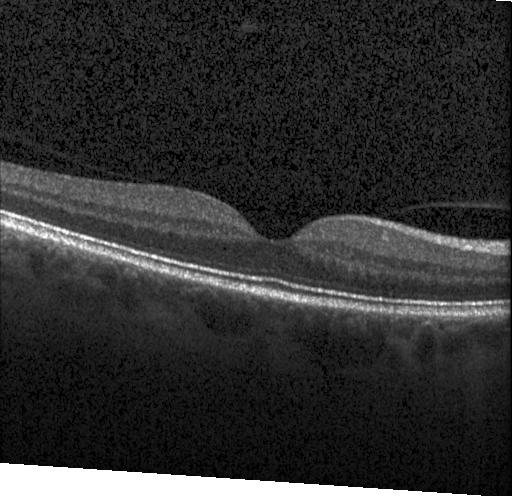 Heidelberg Spectralis; OCT B-scan.
Impression: no CNV, no DME, and no drusen.